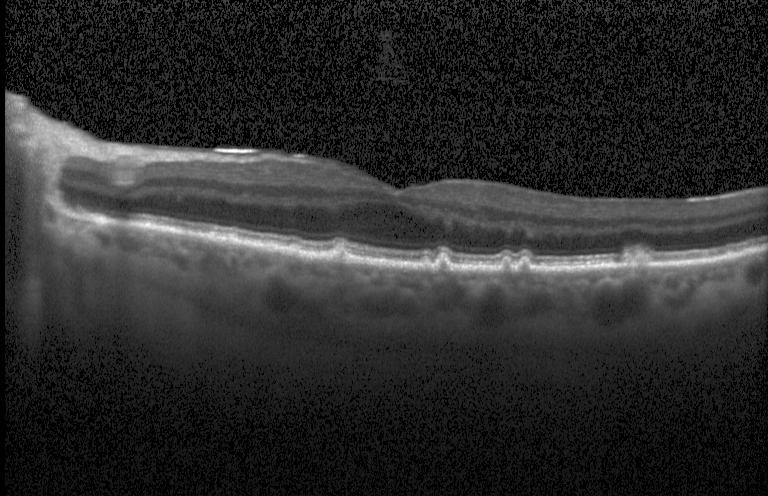

Assessment: multiple drusen.